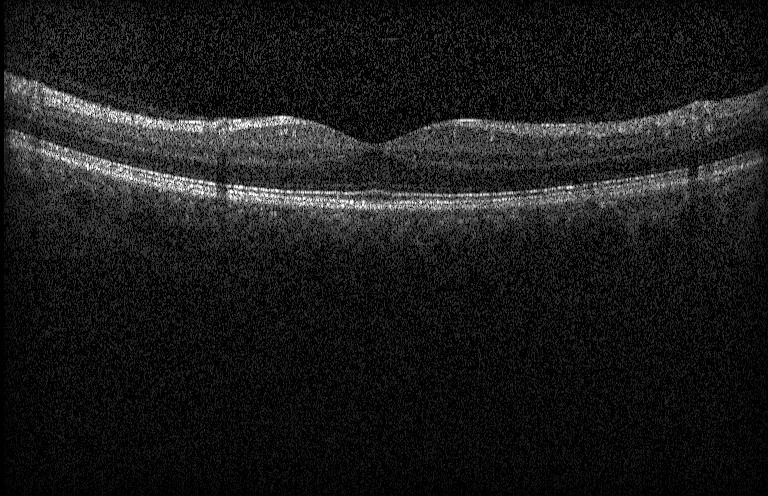
Macular OCT: neither choroidal neovascularization, diabetic macular edema, nor drusen.